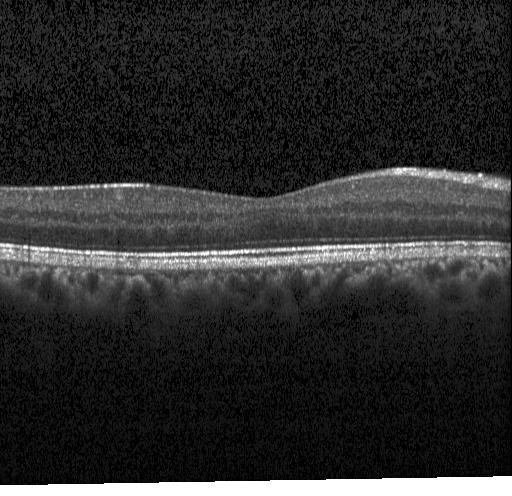
Macular OCT: no evidence of choroidal neovascularization, diabetic macular edema, or drusen.